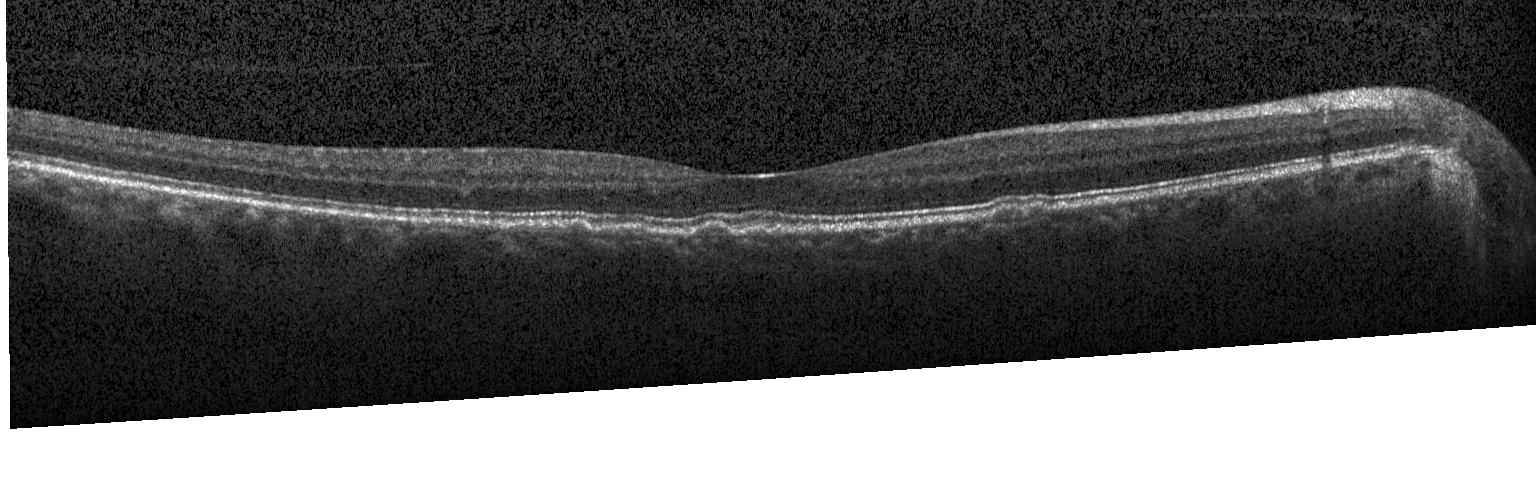 SD-OCT; retinal OCT cross-section; centered on the fovea
Assessment: sub-RPE drusenoid deposits.